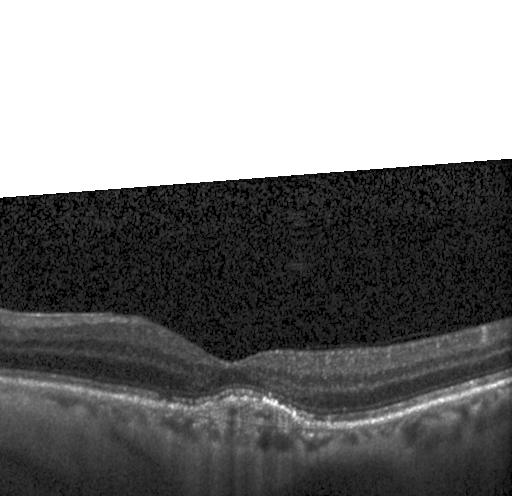
Optical coherence tomography scan
Diagnosis: a choroidal neovascular membrane.